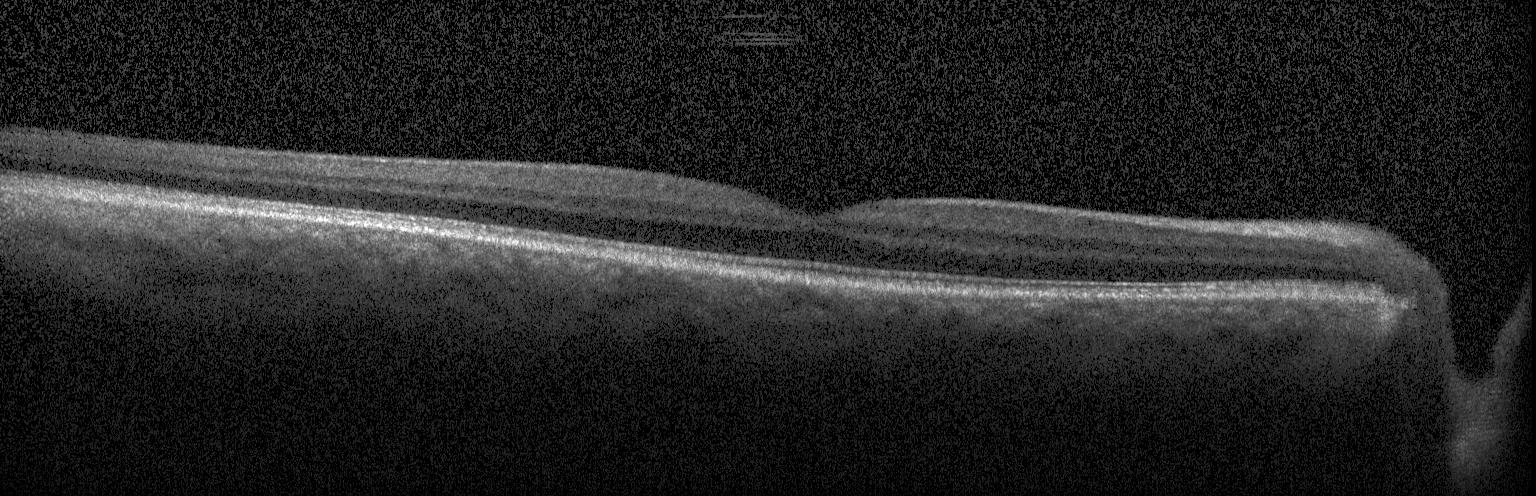

Retinal OCT cross-section · fovea-centered
Neither CNV, DME, nor drusen.